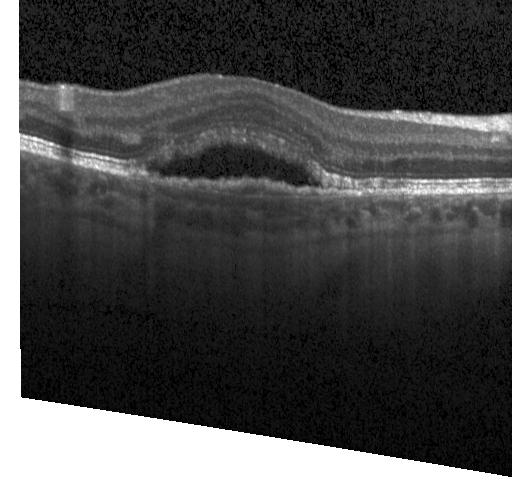

OCT line scan — This B-scan demonstrates choroidal neovascularization.